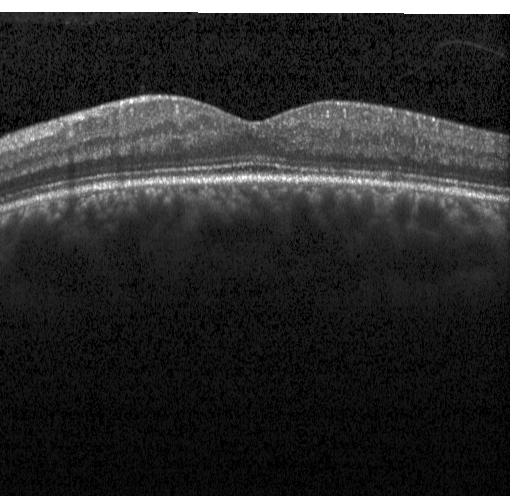
OCT line scan · spectral-domain optical coherence tomography · through the macula. The scan shows no choroidal neovascularization, diabetic macular edema, or drusen.